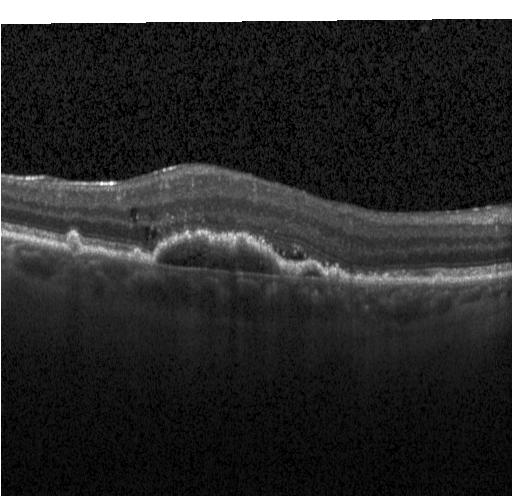

This B-scan demonstrates choroidal neovascularization (CNV).